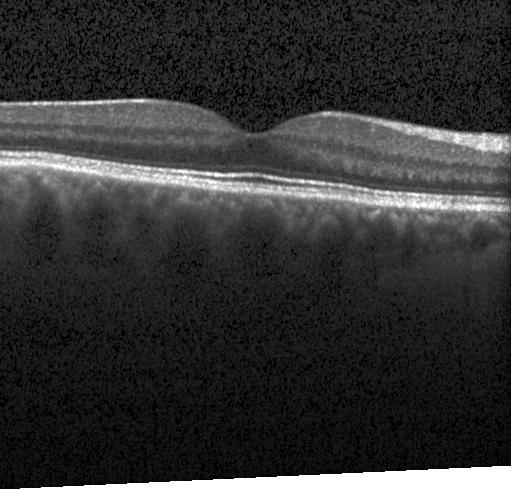 Impression: no CNV, no DME, and no drusen.